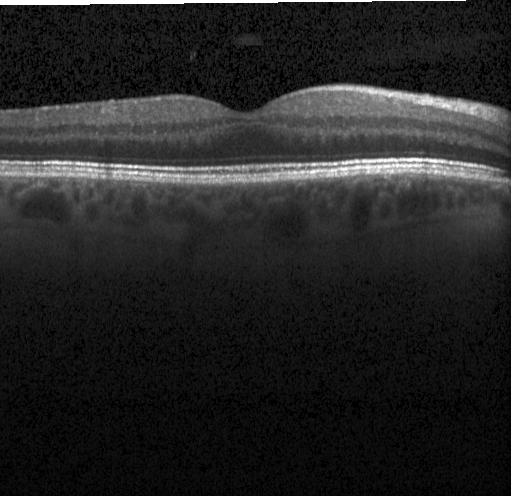

Retinal OCT B-scan. Diagnosis: no evidence of CNV, DME, or drusen.